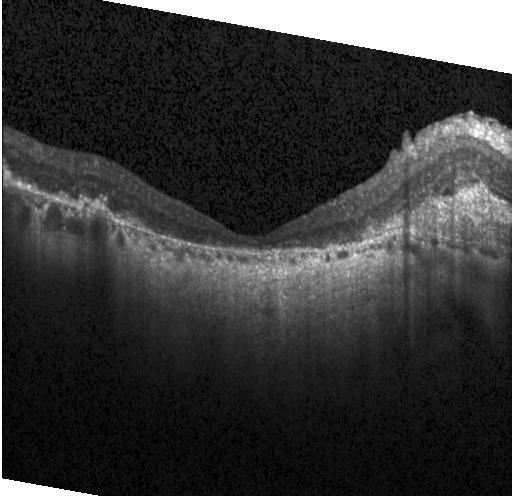

Spectral-domain optical coherence tomography · horizontal scan through the fovea · instrument: Heidelberg Spectralis · optical coherence tomography B-scan — Finding: a choroidal neovascular membrane.